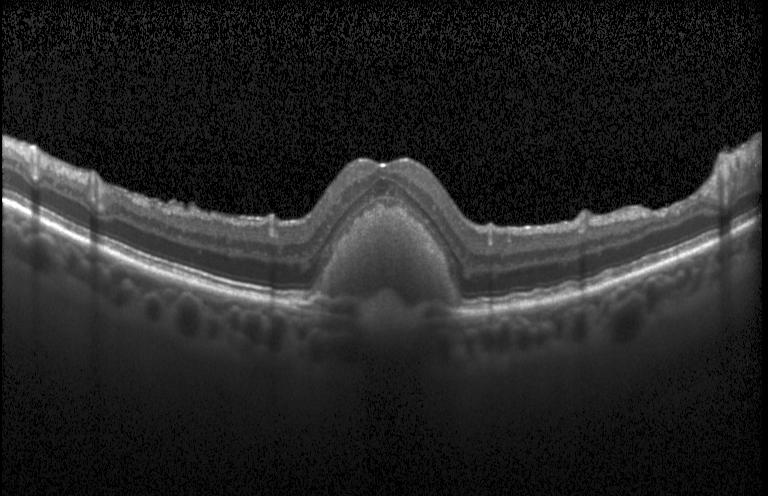 Optical coherence tomography scan. Macular scan.
The scan shows a choroidal neovascular membrane.